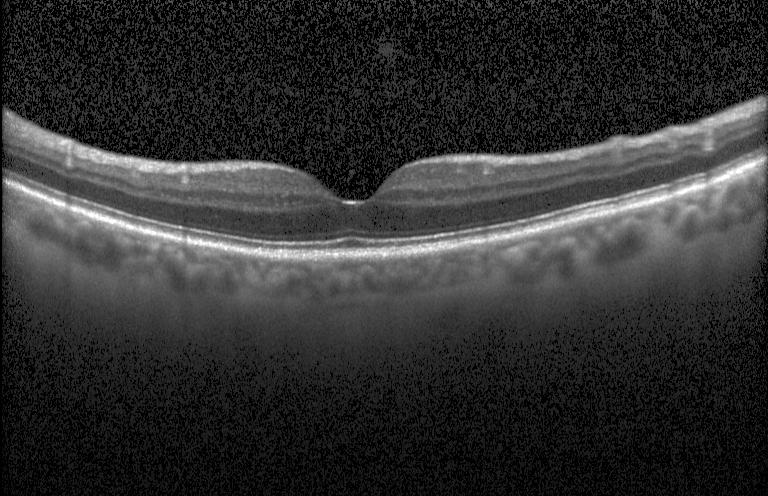 Retinal OCT cross-section · horizontal scan through the fovea.
This B-scan demonstrates no CNV, no DME, and no drusen.